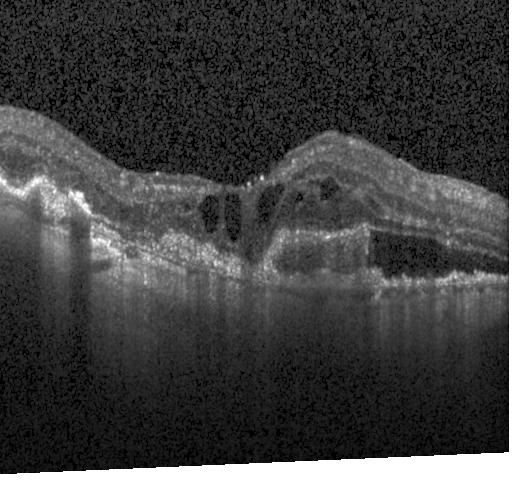
Spectral-domain optical coherence tomography · optical coherence tomography scan · fovea-centered. Assessment: a choroidal neovascular membrane.